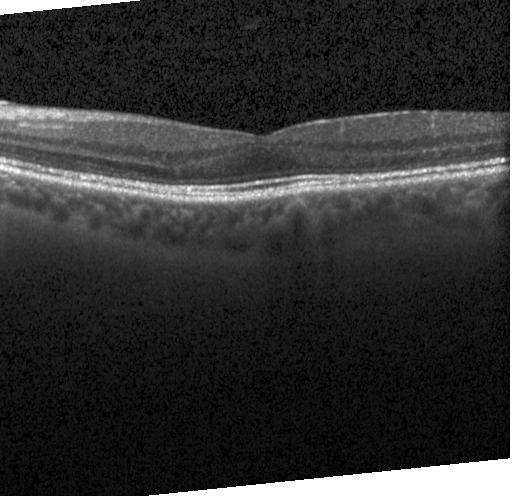

Macular OCT demonstrating no CNV, no DME, and no drusen.